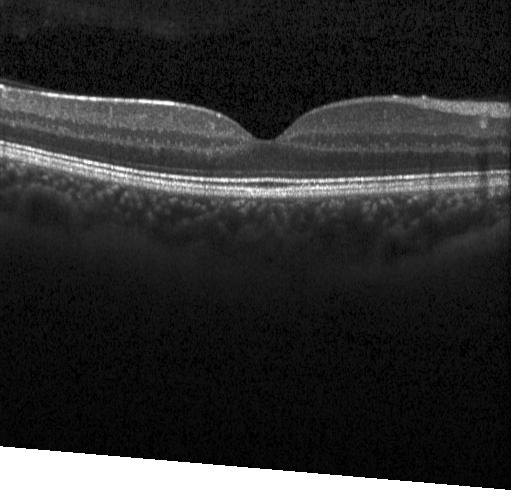

Retinal OCT cross-section.
OCT finding: no evidence of CNV, DME, or drusen.